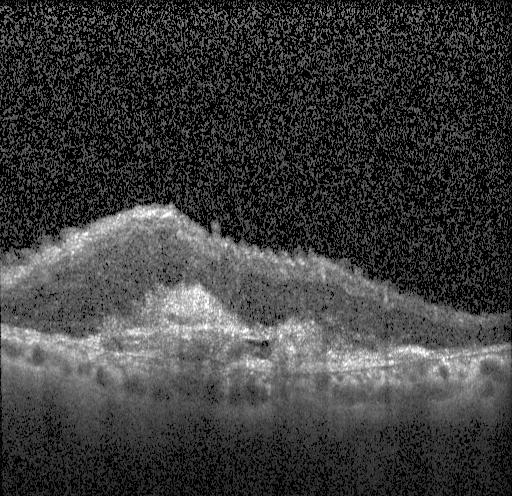 Optical coherence tomography scan. Assessment: choroidal neovascularization (CNV).